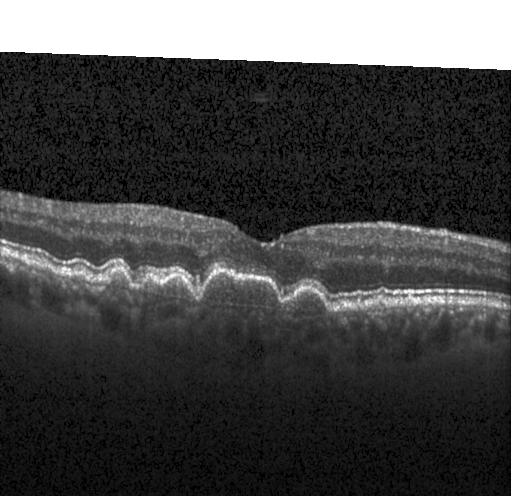 The scan shows sub-RPE drusenoid deposits.